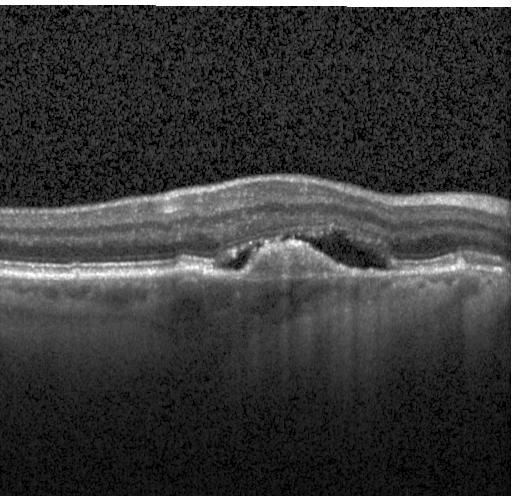 SD-OCT, OCT line scan, fovea-centered, Heidelberg Spectralis OCT system. This B-scan demonstrates a choroidal neovascular membrane.